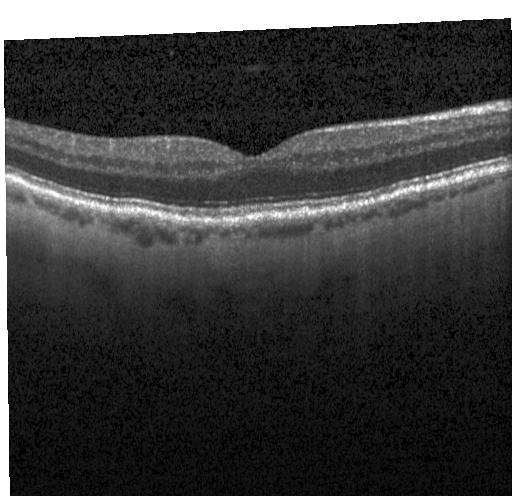

Retinal OCT B-scan · spectral-domain OCT · macular scan · acquired on a Heidelberg Spectralis — Finding: no CNV, DME, or drusen.